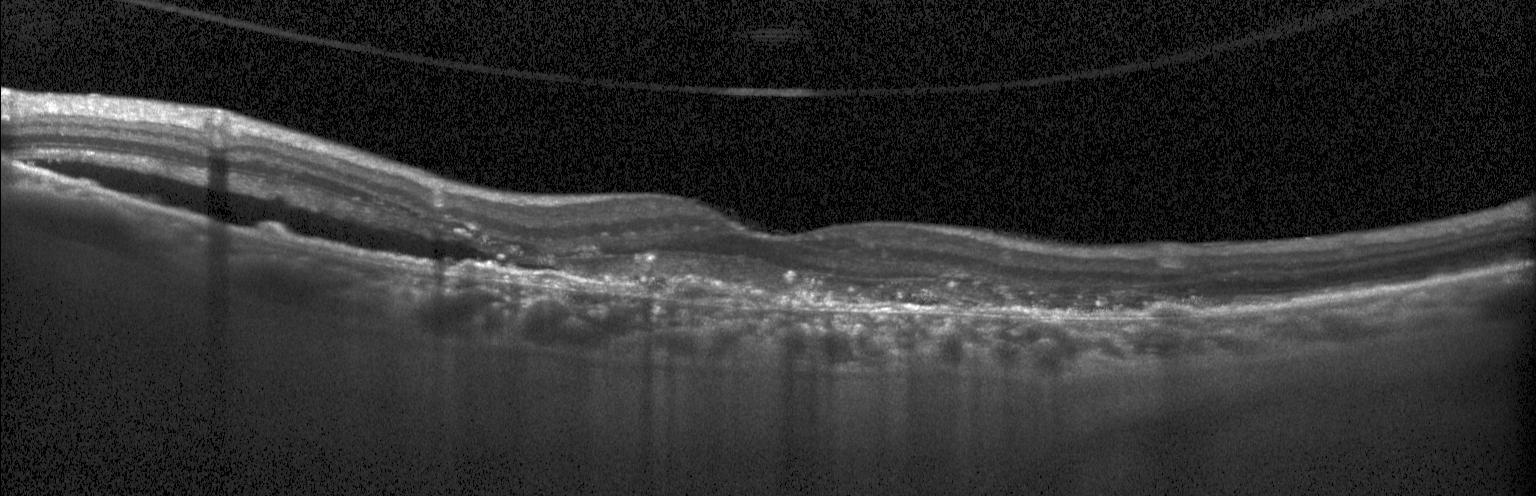

Heidelberg Spectralis OCT system · through the macula · SD-OCT · optical coherence tomography scan. Impression: a choroidal neovascular membrane.